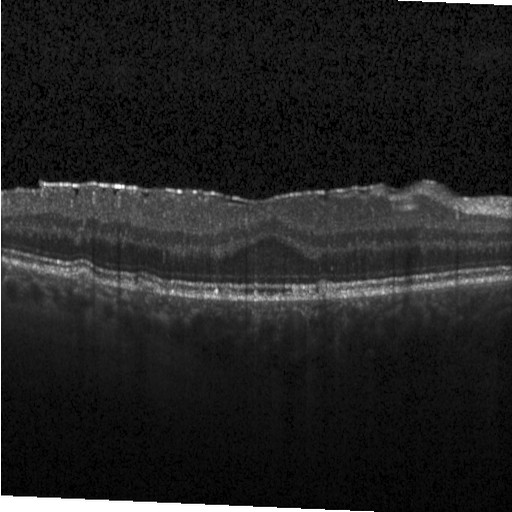

Centered on the fovea. OCT line scan.
Diagnosis: diabetic macular edema (DME).